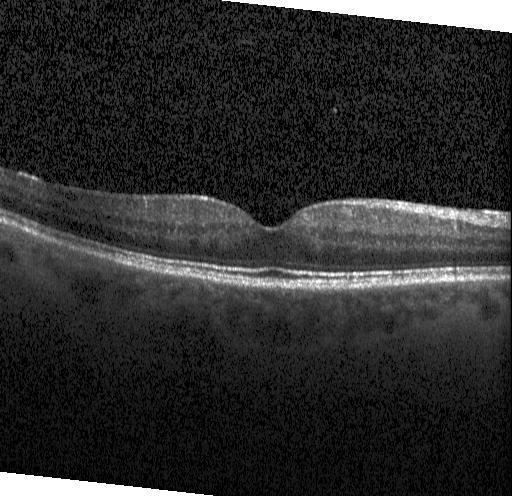
Heidelberg Spectralis OCT system · OCT B-scan · macular scan · spectral-domain OCT.
Assessment: no CNV, no DME, and no drusen.